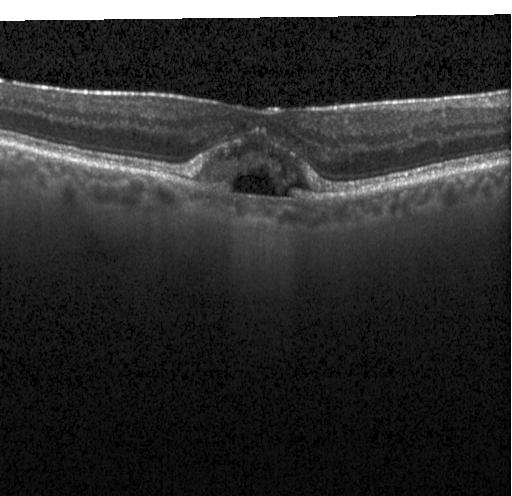 Optical coherence tomography B-scan. Finding: a choroidal neovascular membrane.